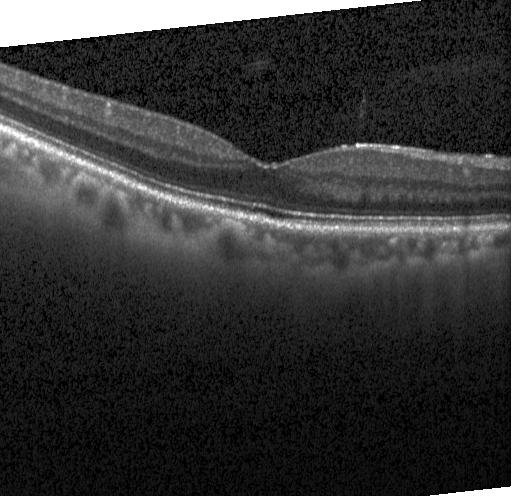
Spectral-domain optical coherence tomography. Retinal OCT cross-section. Instrument: Heidelberg Spectralis — Assessment: no evidence of choroidal neovascularization, diabetic macular edema, or drusen.